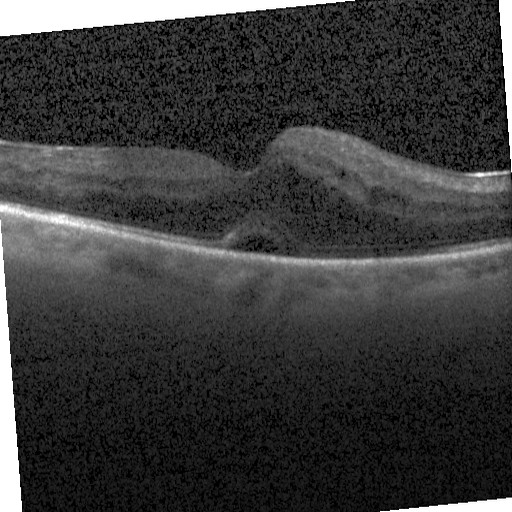

Spectral-domain OCT. OCT line scan. Horizontal scan through the fovea.
Finding: diabetic macular edema.